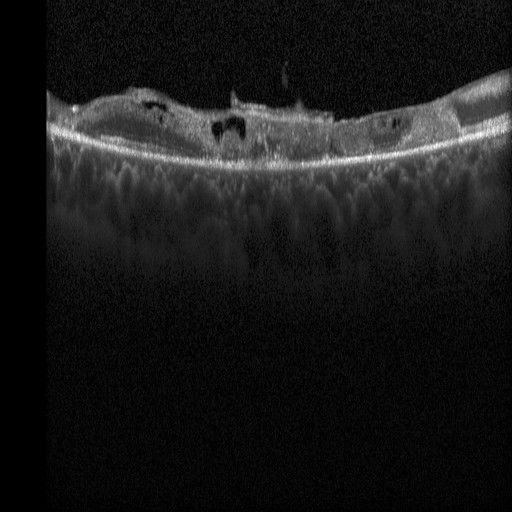 Horizontal scan through the fovea. Instrument: Heidelberg Spectralis. Retinal OCT cross-section. Spectral-domain OCT
Diabetic macular edema (DME).